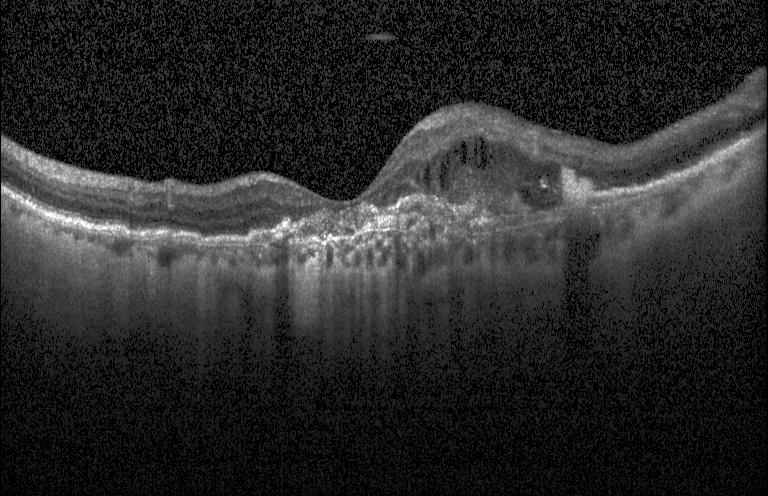

Optical coherence tomography B-scan, Heidelberg Spectralis OCT system, spectral-domain OCT, horizontal scan through the fovea. Diagnosis: CNV.